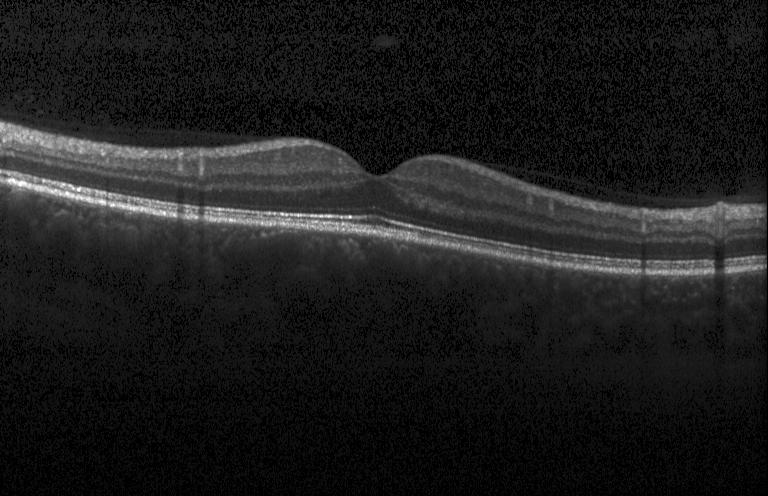
Spectral-domain optical coherence tomography. Centered on the fovea. Instrument: Heidelberg Spectralis. Retinal OCT B-scan
Finding: no choroidal neovascularization, diabetic macular edema, or drusen.